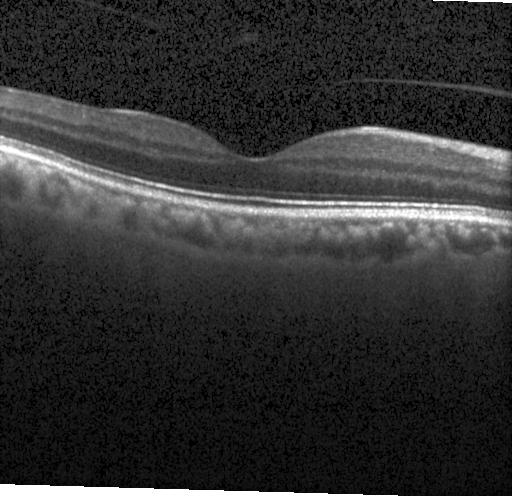

OCT B-scan, through the macula, SD-OCT
The scan shows no CNV, no DME, and no drusen.